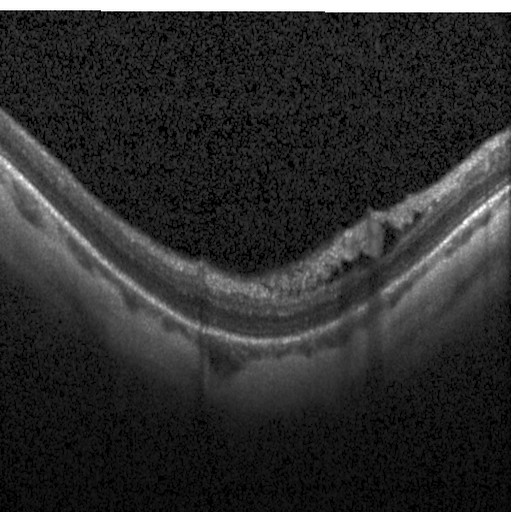
Diagnosis: diabetic macular edema (DME).